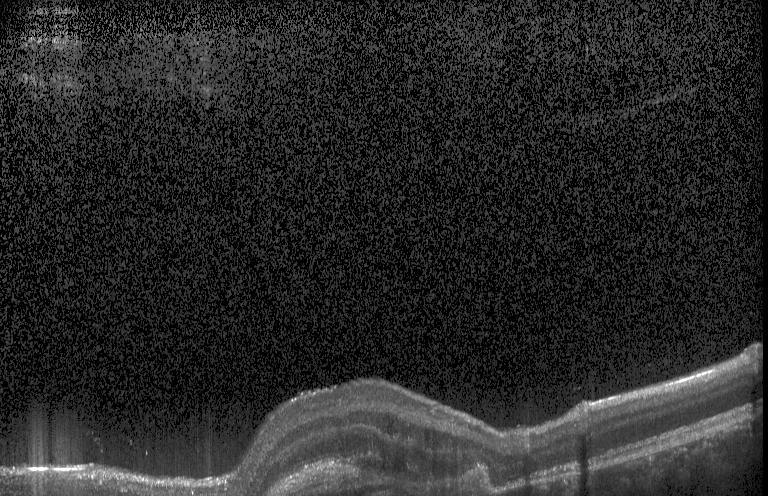 Assessment: a choroidal neovascular membrane.